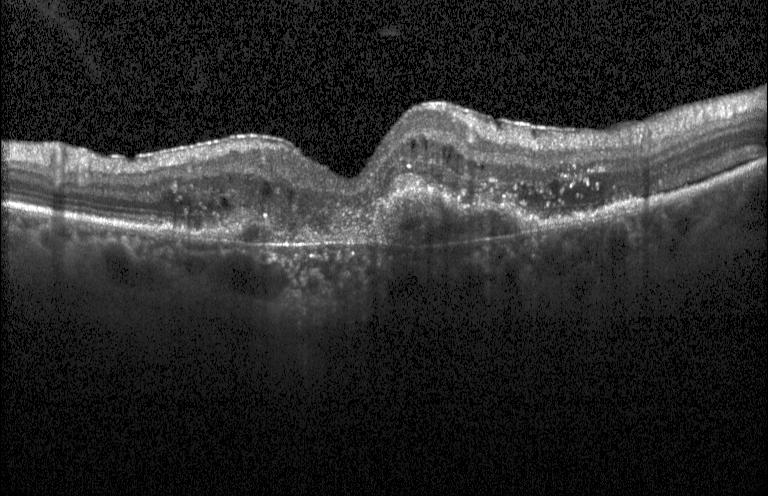
Macular scan, optical coherence tomography B-scan, spectral-domain optical coherence tomography, Heidelberg Spectralis
Finding: a choroidal neovascular membrane.